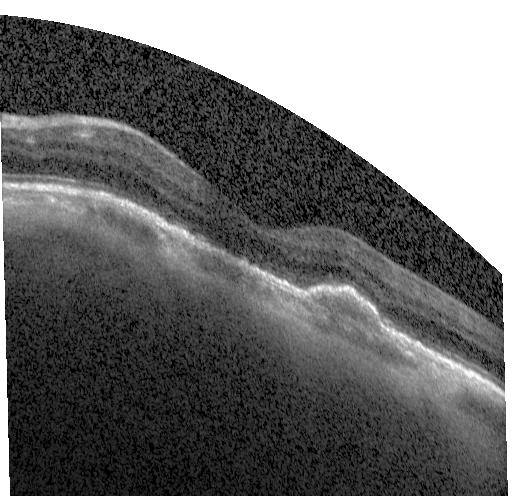 Optical coherence tomography B-scan. Macular scan. Spectral-domain optical coherence tomography. Heidelberg Spectralis.
Choroidal neovascularization (CNV).